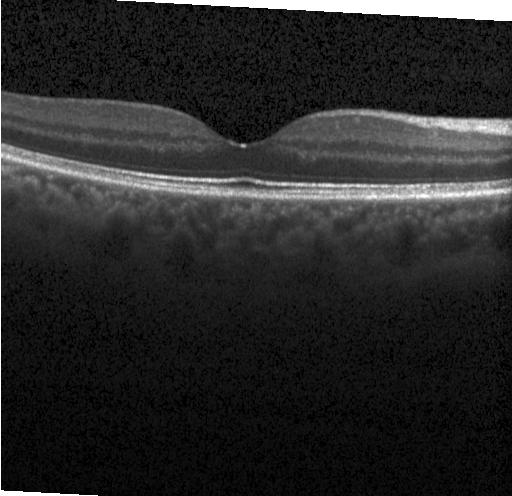 Retinal OCT cross-section · spectral-domain optical coherence tomography · acquired on a Heidelberg Spectralis · fovea-centered — The scan shows no choroidal neovascularization, diabetic macular edema, or drusen.